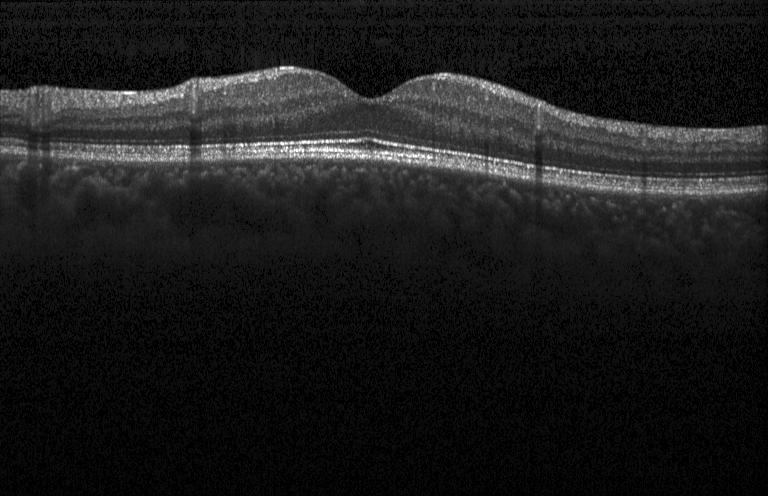
Centered on the fovea, OCT line scan, Heidelberg Spectralis OCT system, SD-OCT. Diagnosis: no evidence of CNV, DME, or drusen.